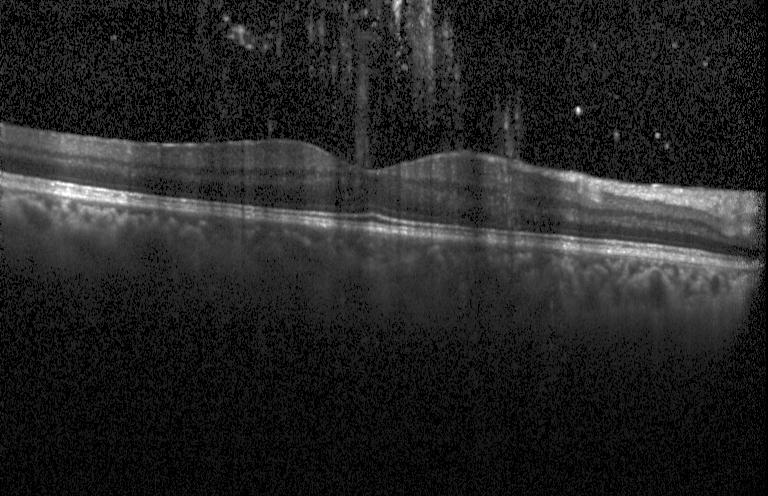
Retinal OCT cross-section showing no choroidal neovascularization, no diabetic macular edema, and no drusen.